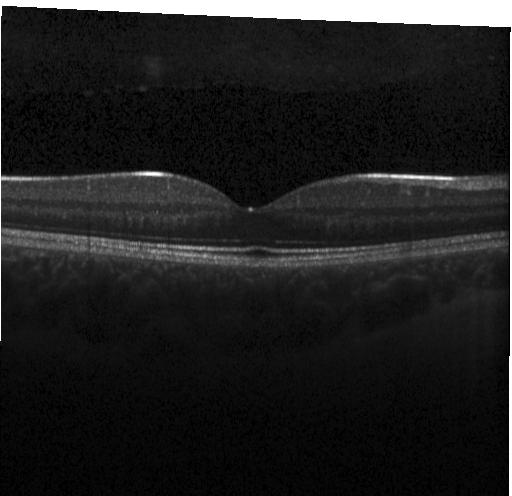
Horizontal scan through the fovea · retinal OCT B-scan · Heidelberg Spectralis — Diagnosis: neither CNV, DME, nor drusen.